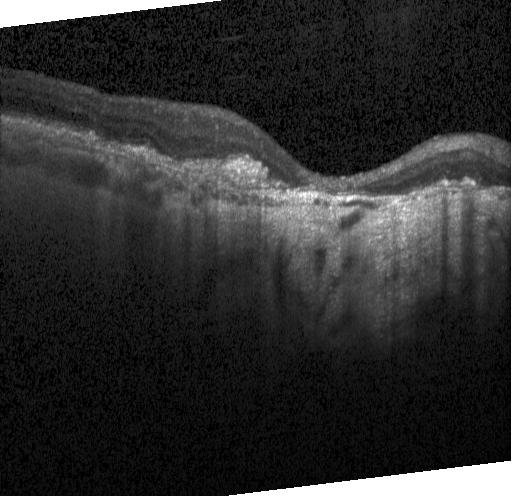

Retinal OCT B-scan, through the macula, acquired on a Heidelberg Spectralis — CNV.